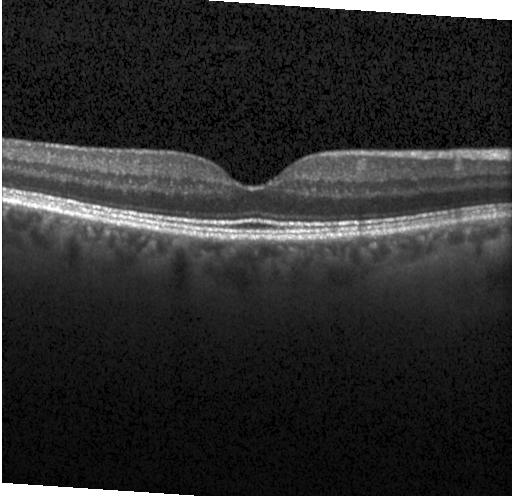 Fovea-centered · retinal OCT B-scan — Macular OCT: no evidence of choroidal neovascularization, diabetic macular edema, or drusen.